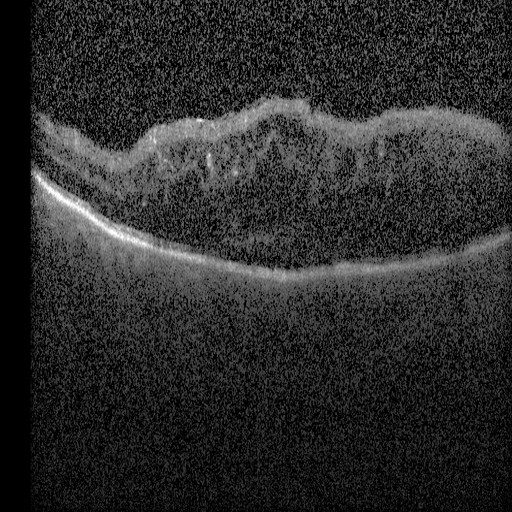

Dx: diabetic macular edema.